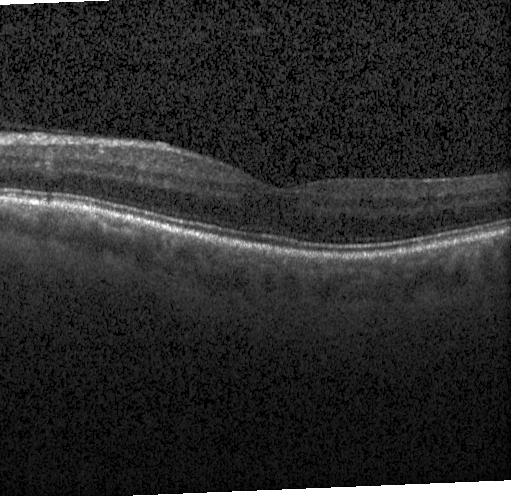

OCT line scan, SD-OCT, Heidelberg Spectralis, macular scan. Impression: no evidence of choroidal neovascularization, diabetic macular edema, or drusen.